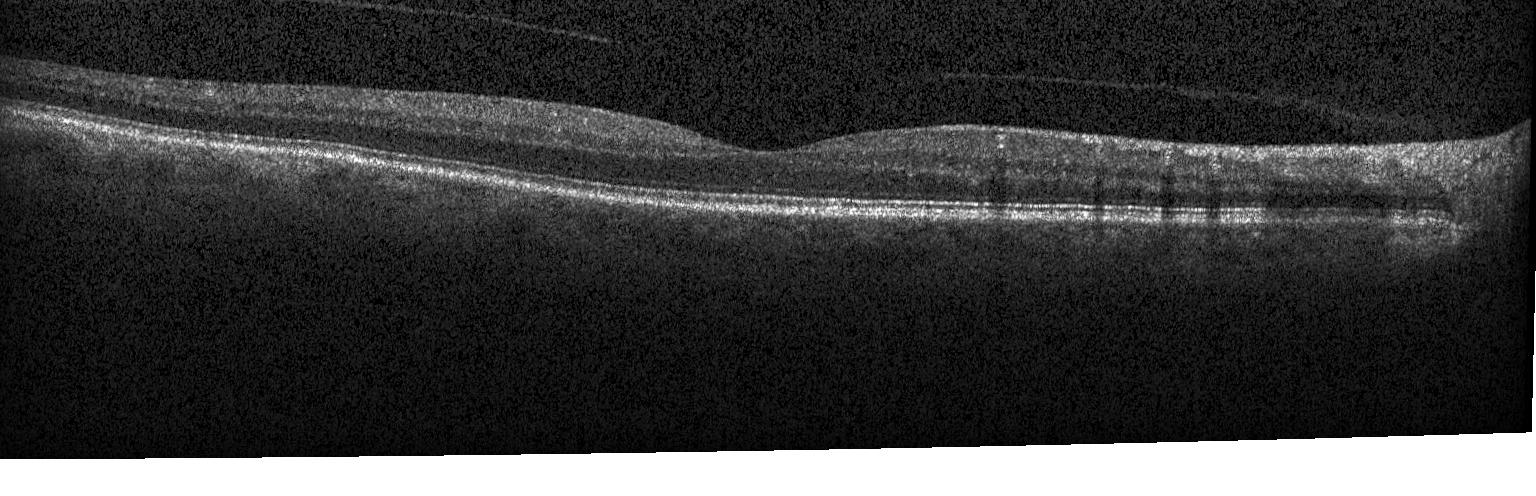

Optical coherence tomography B-scan — Impression: no choroidal neovascularization, no diabetic macular edema, and no drusen.